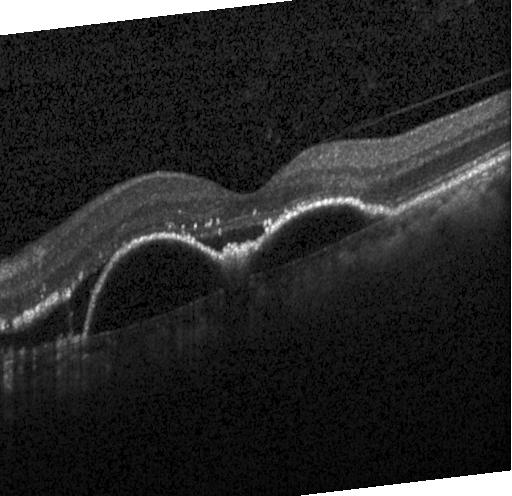 Spectral-domain OCT B-scan: a choroidal neovascular membrane.